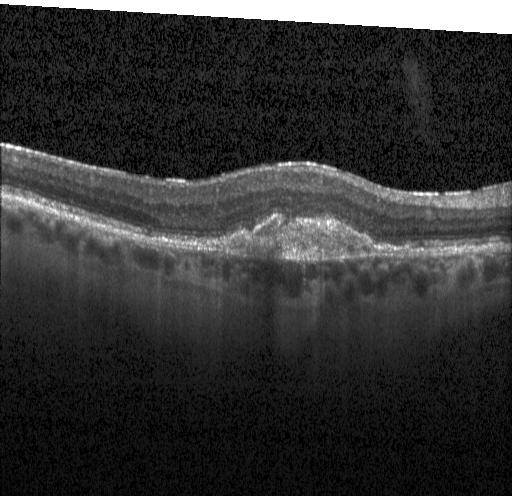
OCT B-scan showing a choroidal neovascular membrane.